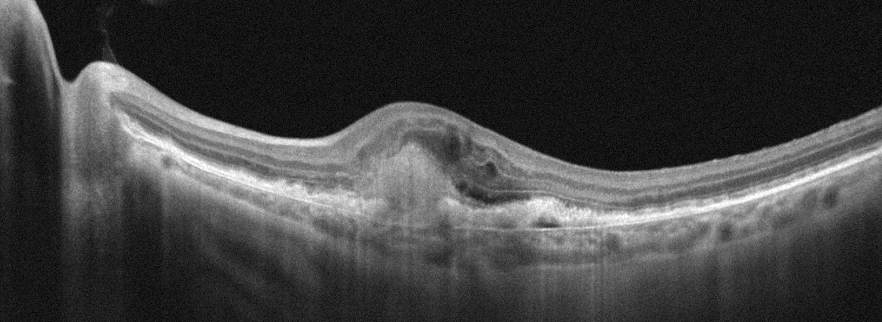

Retinal OCT cross-section · fovea-centered · acquired on an Optovue Avanti RTVue XR. The scan shows age-related macular degeneration.